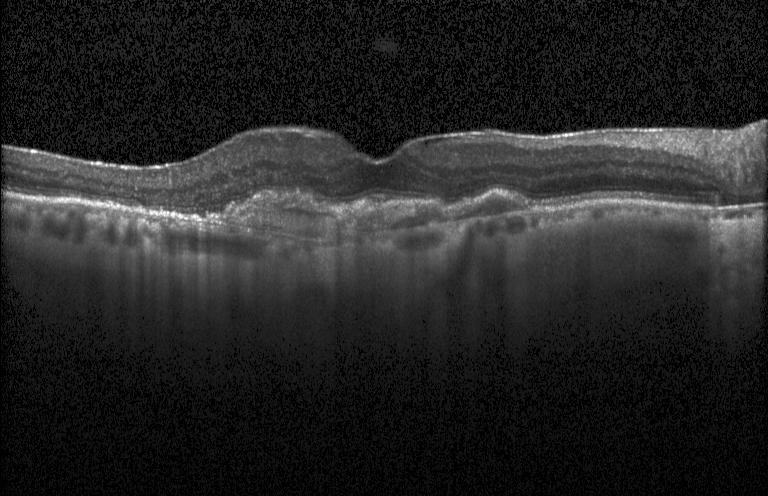
Impression: a choroidal neovascular membrane.